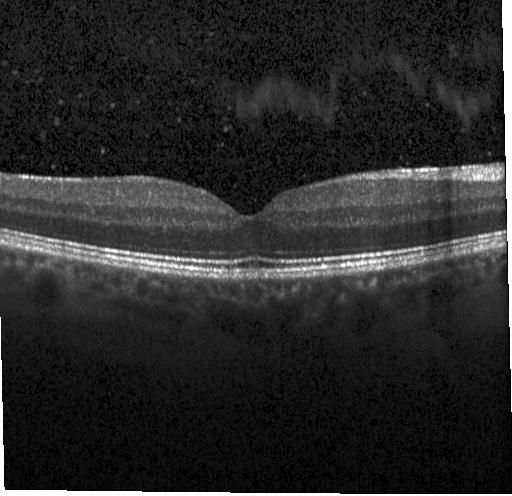

Dx: no evidence of CNV, DME, or drusen.